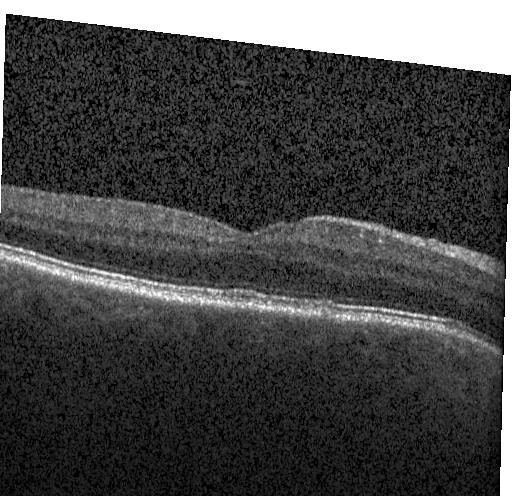 Diagnosis: no CNV, no DME, and no drusen.